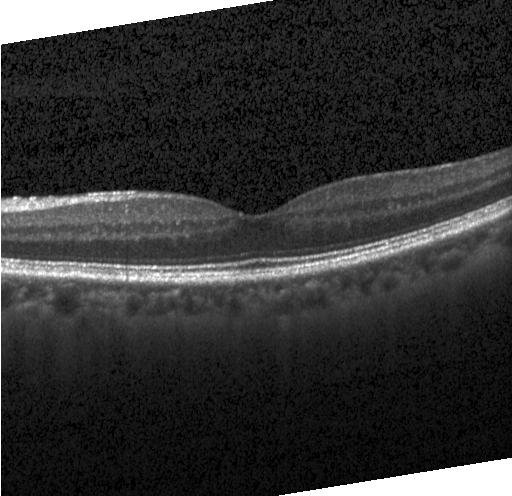
Diagnosis: neither CNV, DME, nor drusen.